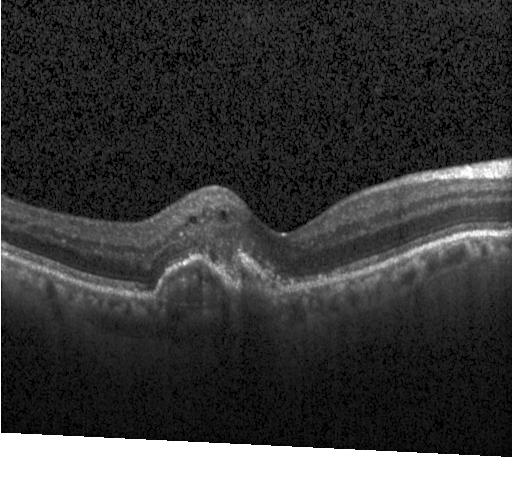

Retinal OCT B-scan.
Macular OCT: choroidal neovascularization.